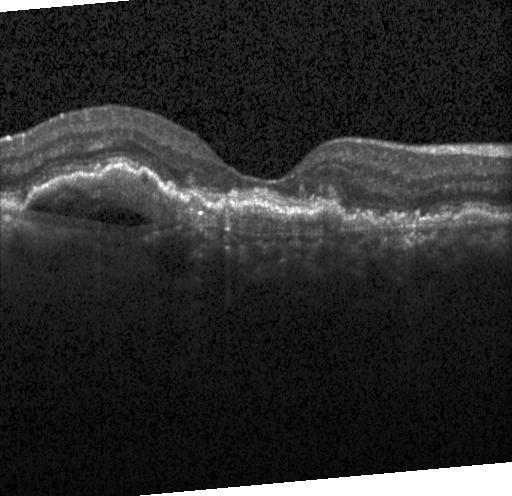 Diagnosis: choroidal neovascularization.